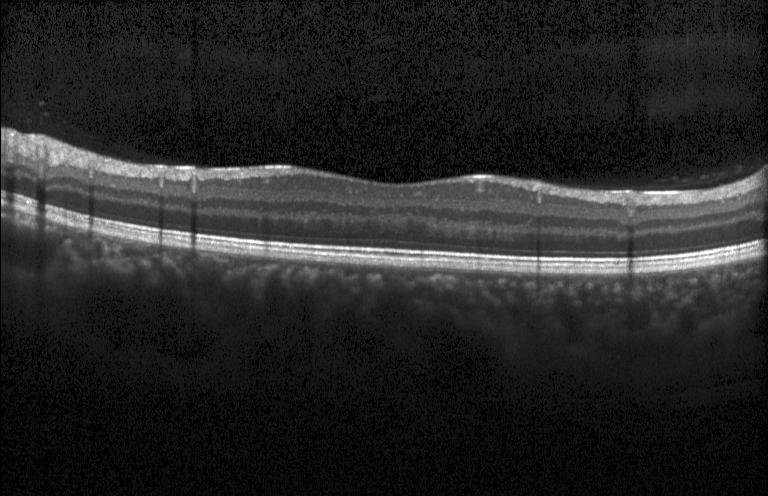

Impression: neither choroidal neovascularization, diabetic macular edema, nor drusen.